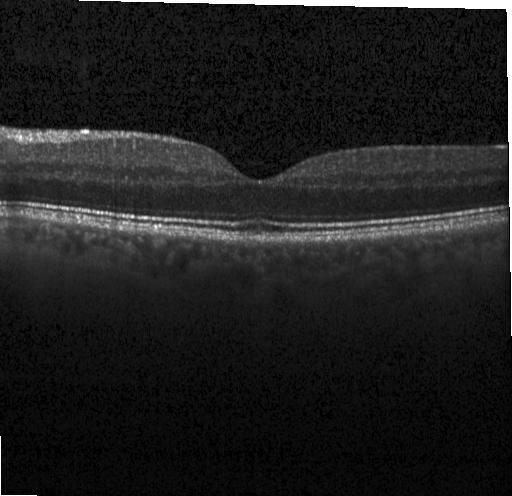
Retinal OCT cross-section
Diagnosis: no choroidal neovascularization, diabetic macular edema, or drusen.